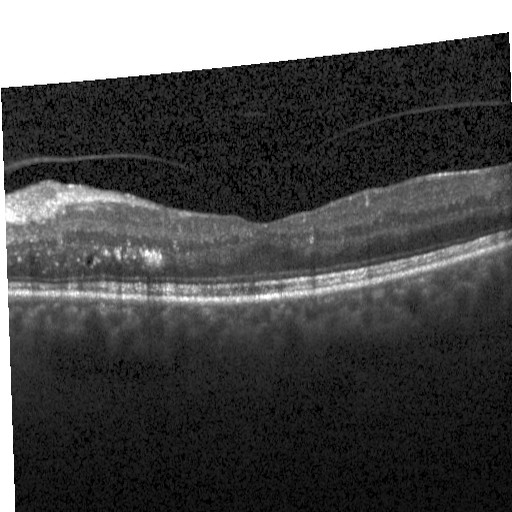
OCT scan showing diabetic macular edema.